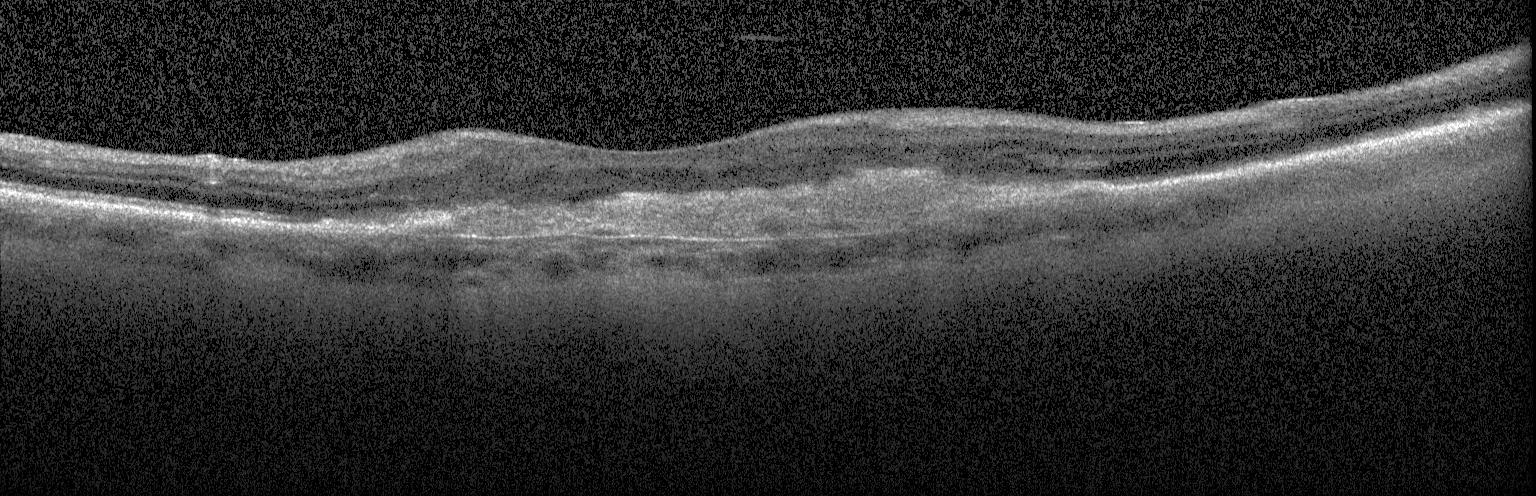 Acquired on a Heidelberg Spectralis, spectral-domain optical coherence tomography, retinal OCT cross-section, through the macula
A choroidal neovascular membrane.